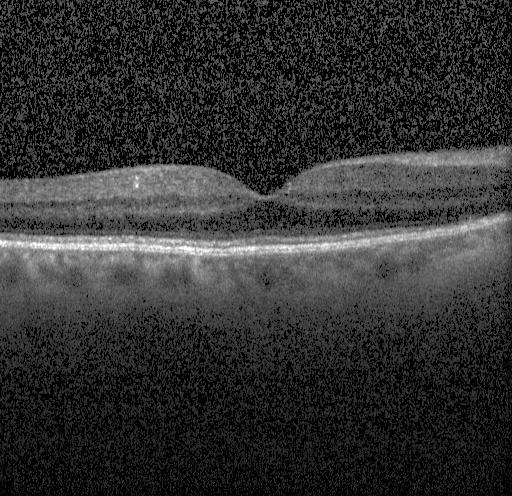
Retinal OCT B-scan — Assessment: no evidence of choroidal neovascularization, diabetic macular edema, or drusen.